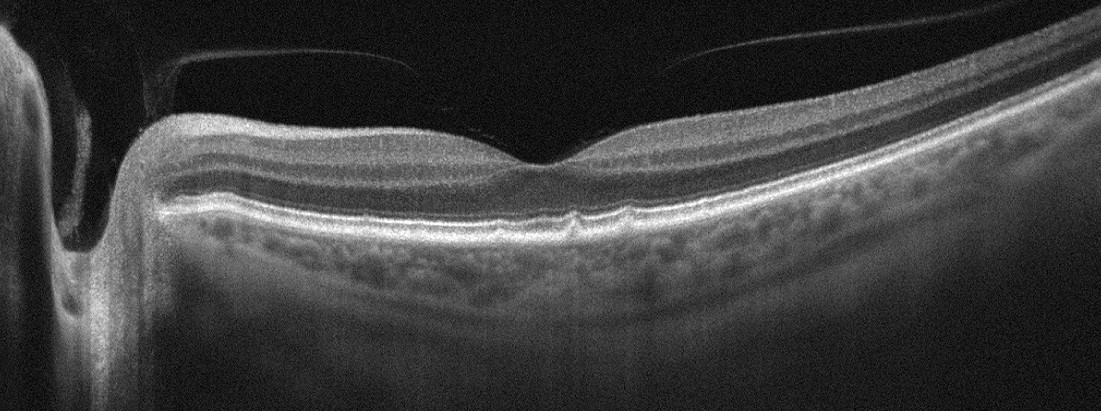
Retinal OCT B-scan.
OCT finding: age-related macular degeneration.